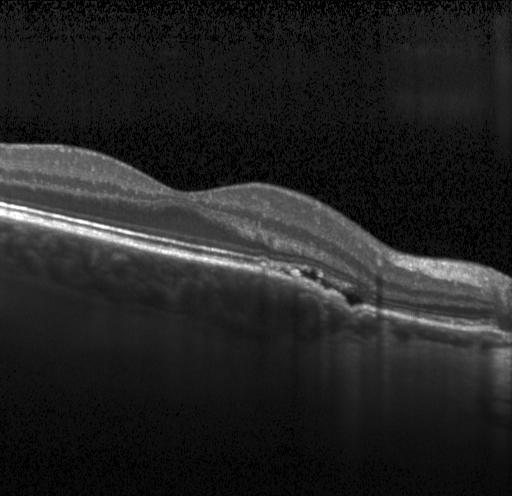

OCT B-scan, through the macula.
Finding: a choroidal neovascular membrane.